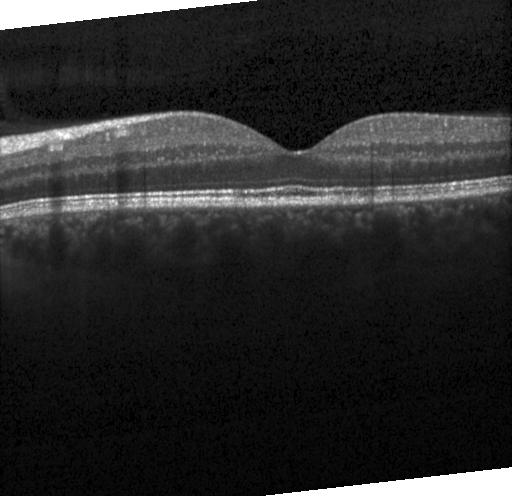
OCT B-scan
The scan shows no choroidal neovascularization, diabetic macular edema, or drusen.